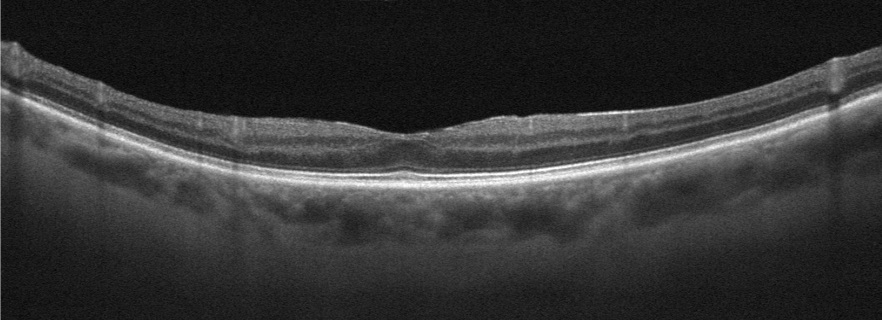
OCT finding: epiretinal membrane (ERM).